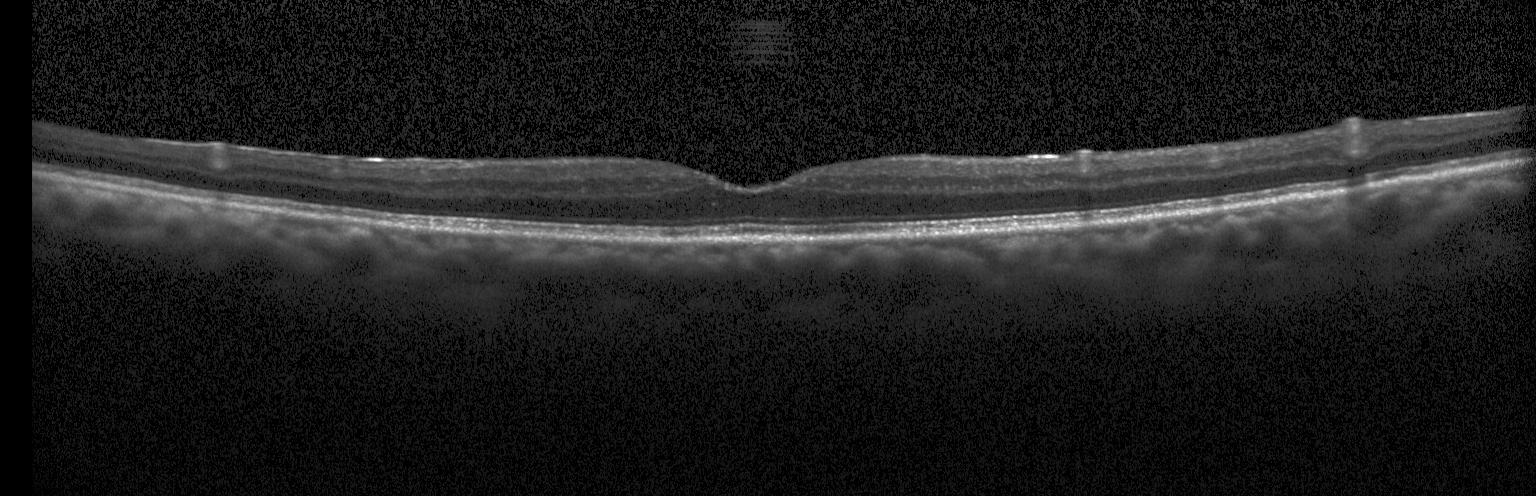 Optical coherence tomography scan, through the macula, Heidelberg Spectralis OCT system.
Diagnosis: no choroidal neovascularization, no diabetic macular edema, and no drusen.